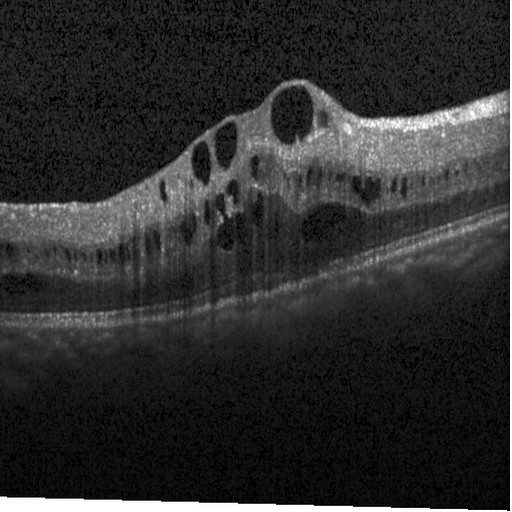
Retinal OCT B-scan, acquired on a Heidelberg Spectralis. Macular OCT: diabetic macular edema (DME).